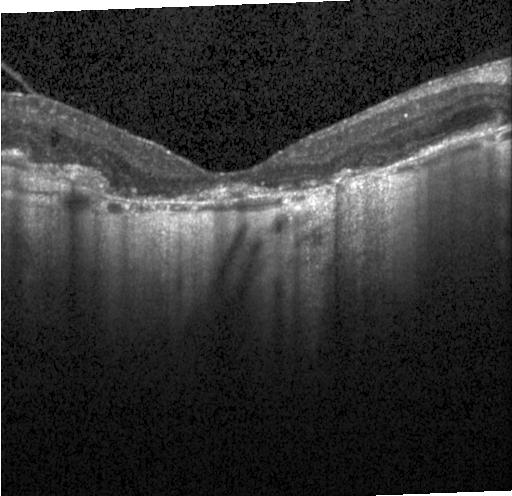
Impression: choroidal neovascularization (CNV).